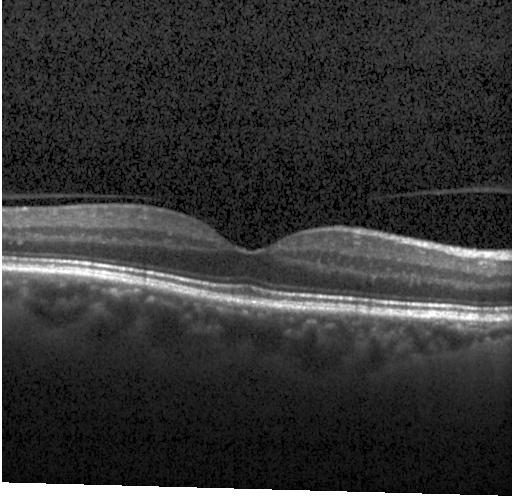 Heidelberg Spectralis. Fovea-centered. Optical coherence tomography scan. The scan shows neither choroidal neovascularization, diabetic macular edema, nor drusen.